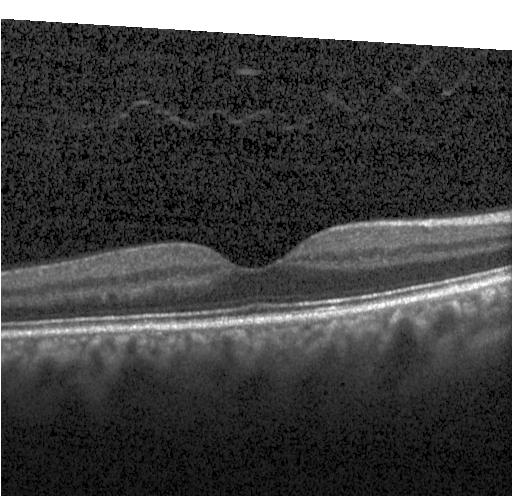

Impression: no evidence of CNV, DME, or drusen.